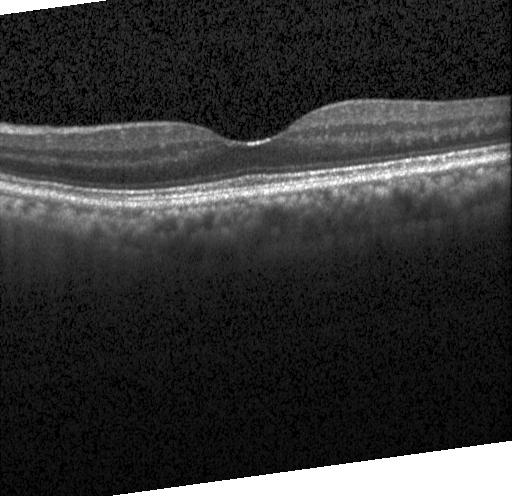

Fovea-centered · instrument: Heidelberg Spectralis · retinal OCT cross-section · SD-OCT. No choroidal neovascularization, diabetic macular edema, or drusen.